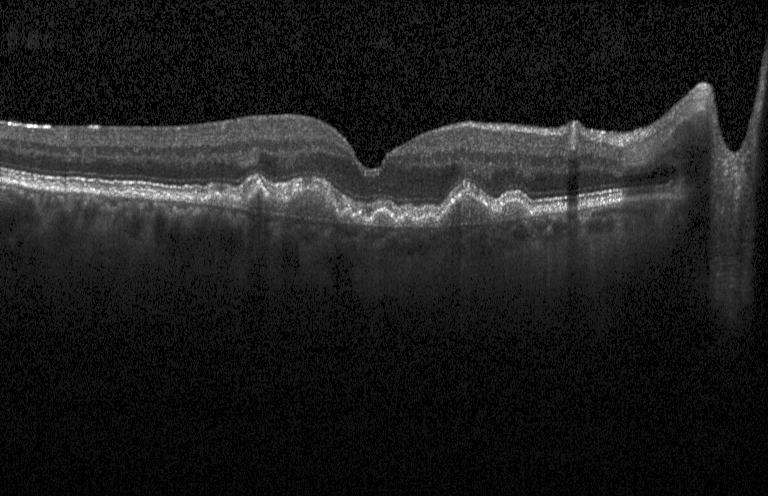
SD-OCT · Heidelberg Spectralis · through the macula · optical coherence tomography B-scan. Assessment: multiple drusen.